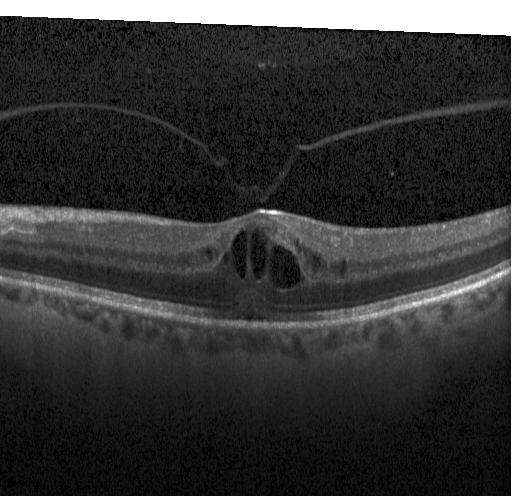
Assessment: DME.